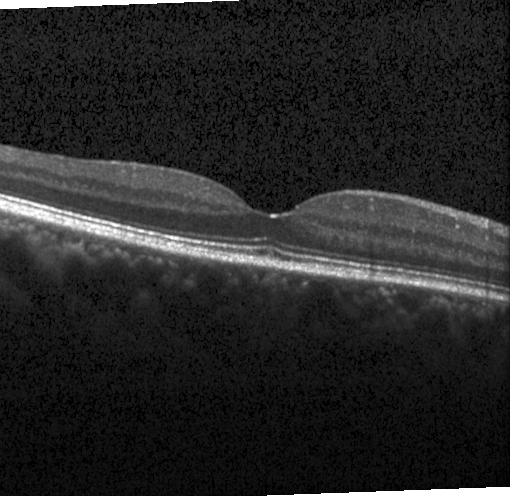
Diagnosis: no CNV, DME, or drusen.